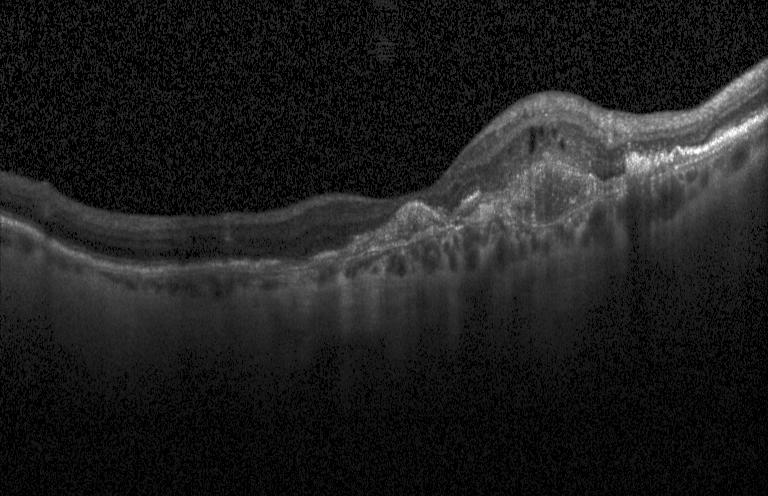

Finding: choroidal neovascularization (CNV).